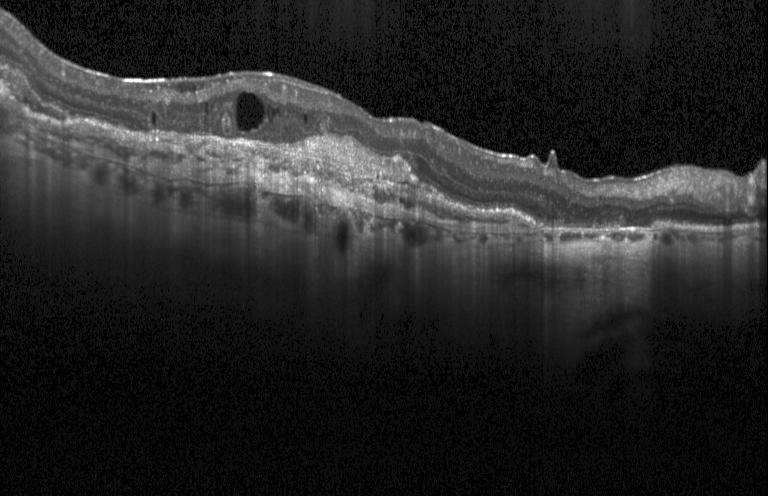

Spectral-domain OCT. Heidelberg Spectralis. OCT line scan. Through the macula.
Diagnosis: a choroidal neovascular membrane.